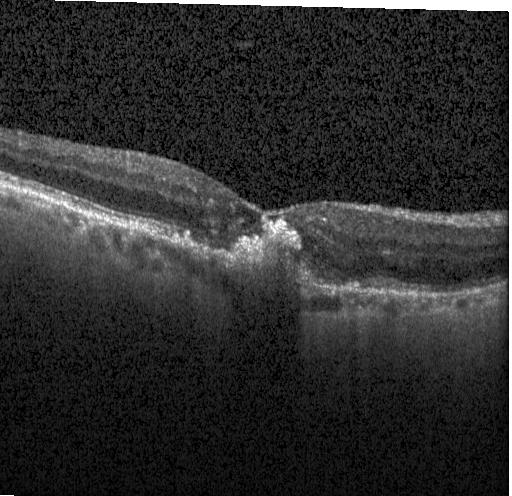 Finding: a choroidal neovascular membrane.